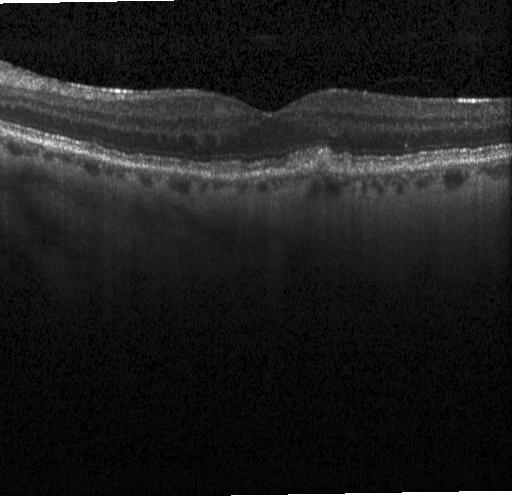 This B-scan demonstrates sub-RPE drusenoid deposits.